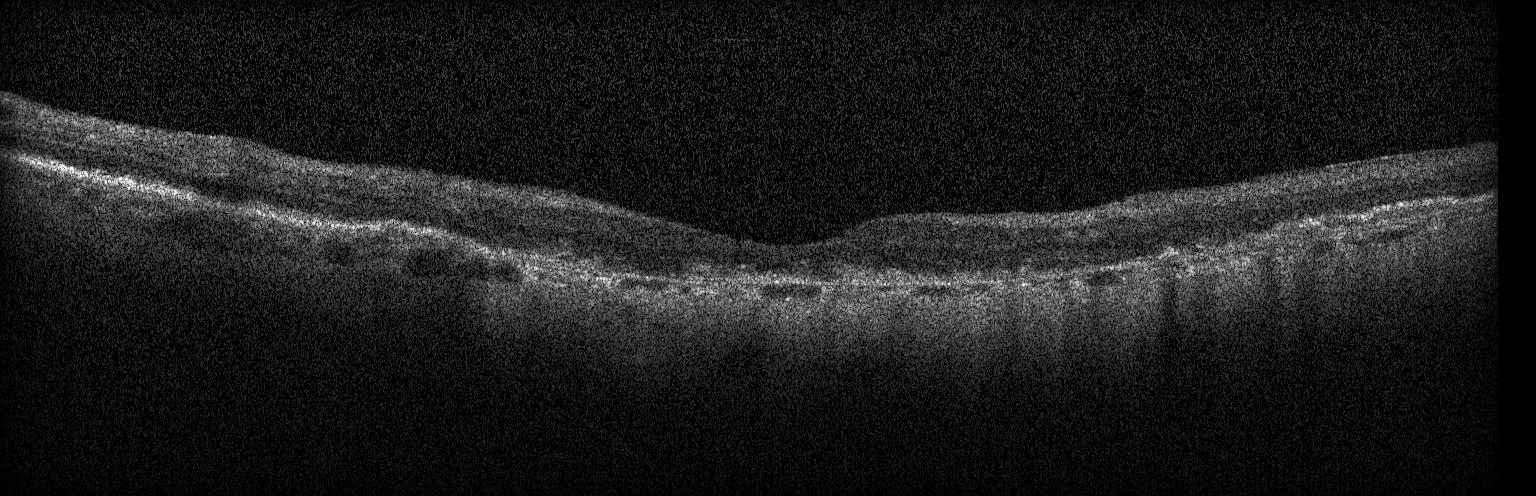

OCT line scan. Finding: a choroidal neovascular membrane.